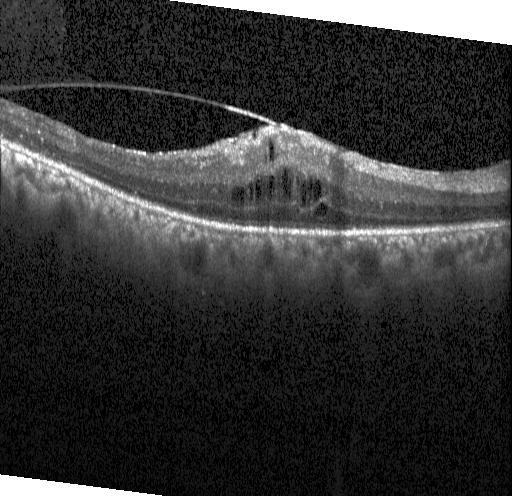
Through the macula, instrument: Heidelberg Spectralis, spectral-domain optical coherence tomography, OCT B-scan
Impression: DME.